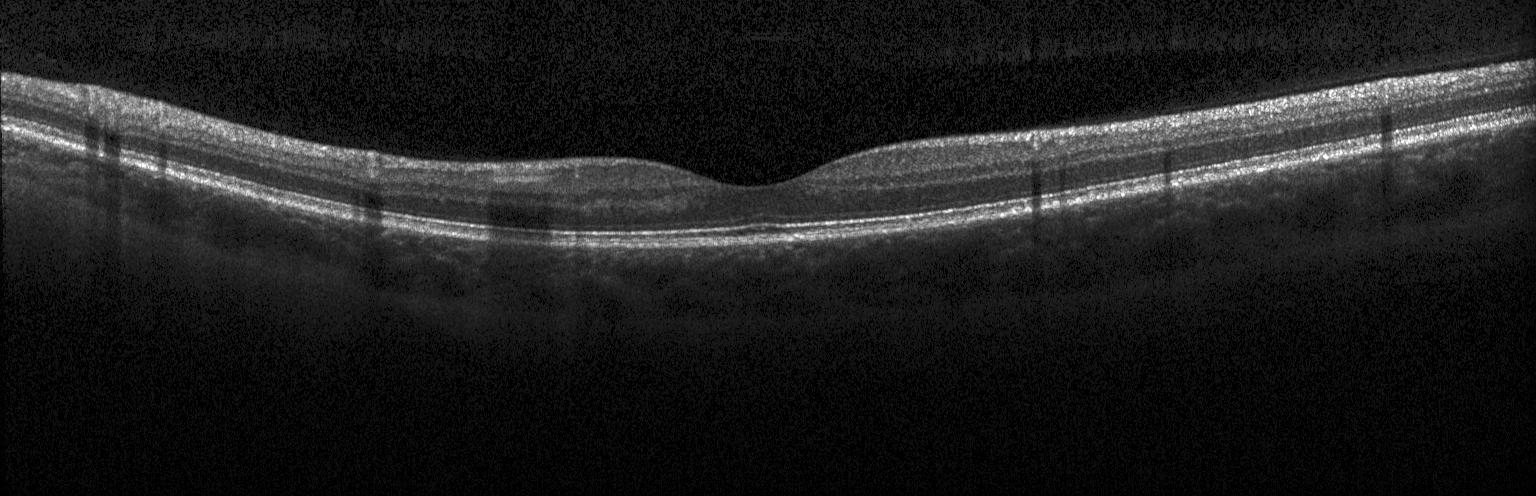

OCT finding: no evidence of CNV, DME, or drusen.